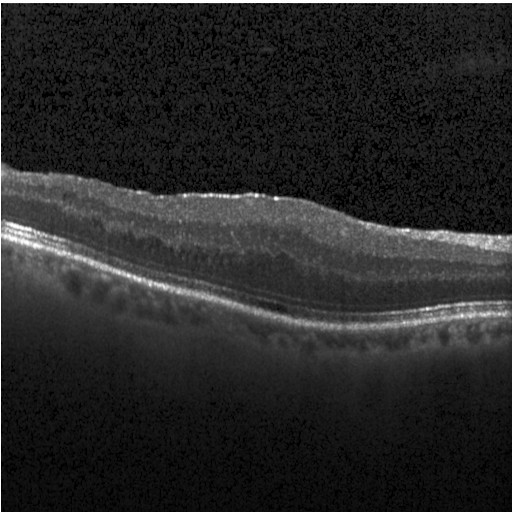

OCT line scan.
Impression: diabetic macular edema.